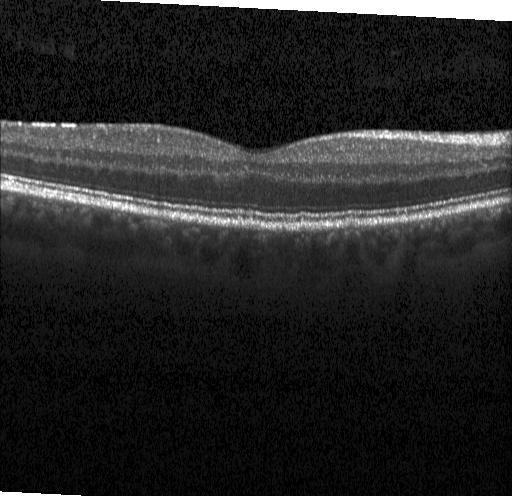 This B-scan demonstrates no CNV, DME, or drusen.